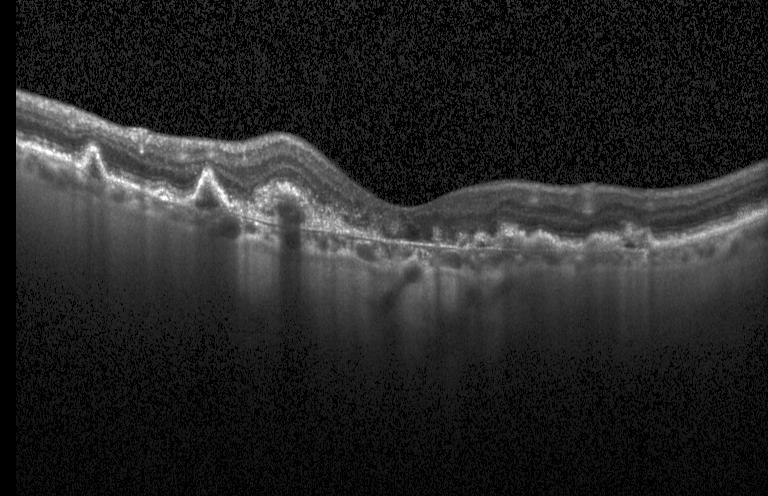

Retinal OCT cross-section, centered on the fovea.
Finding: a choroidal neovascular membrane.